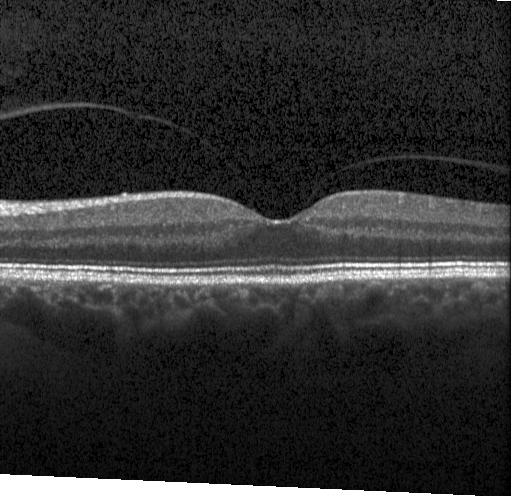

Assessment: neither CNV, DME, nor drusen.